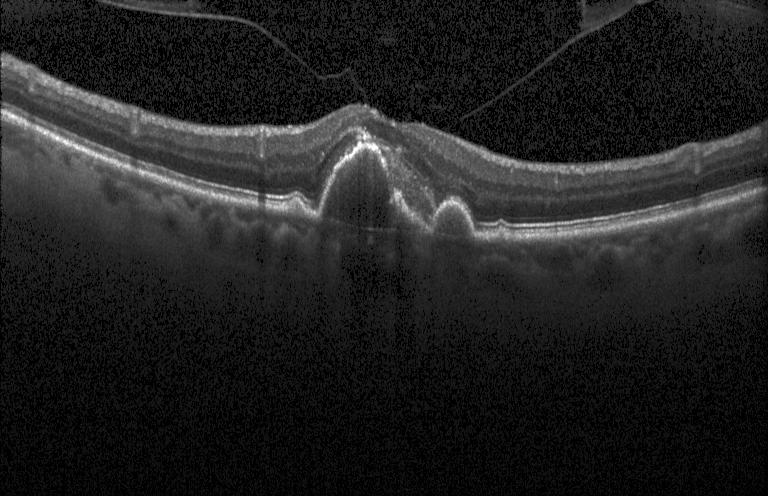 Optical coherence tomography B-scan — Impression: choroidal neovascularization (CNV).